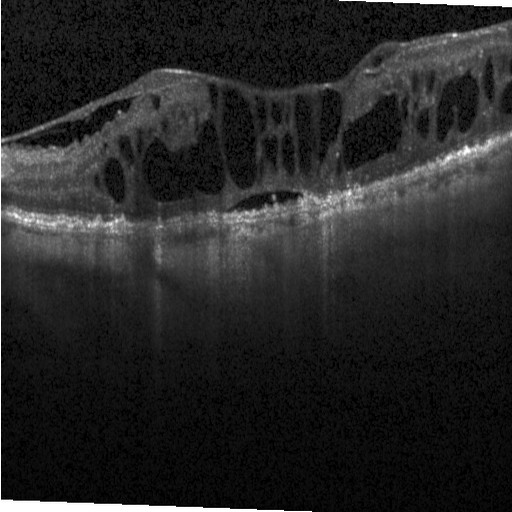

Optical coherence tomography scan
Diabetic macular edema.